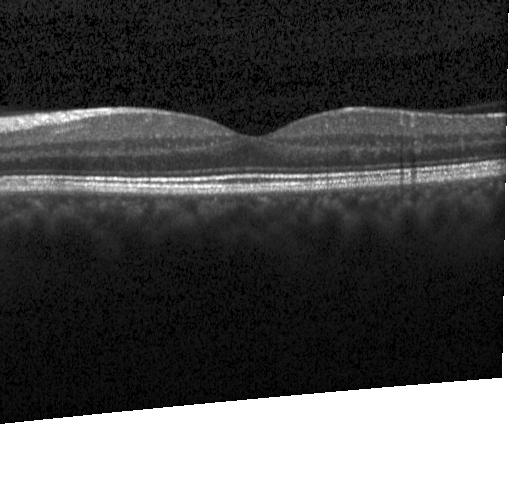
Horizontal scan through the fovea · retinal OCT B-scan
OCT finding: neither choroidal neovascularization, diabetic macular edema, nor drusen.